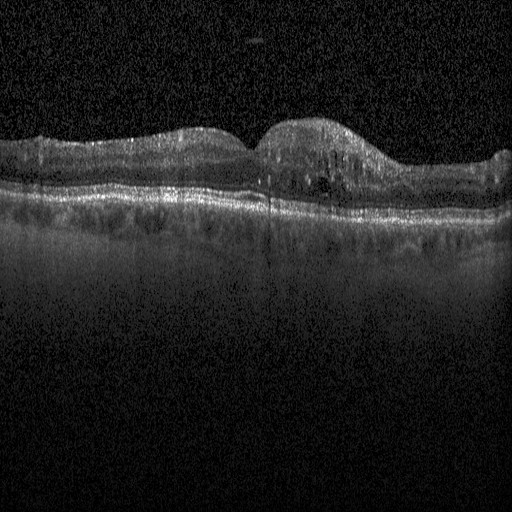

OCT finding: diabetic macular edema.